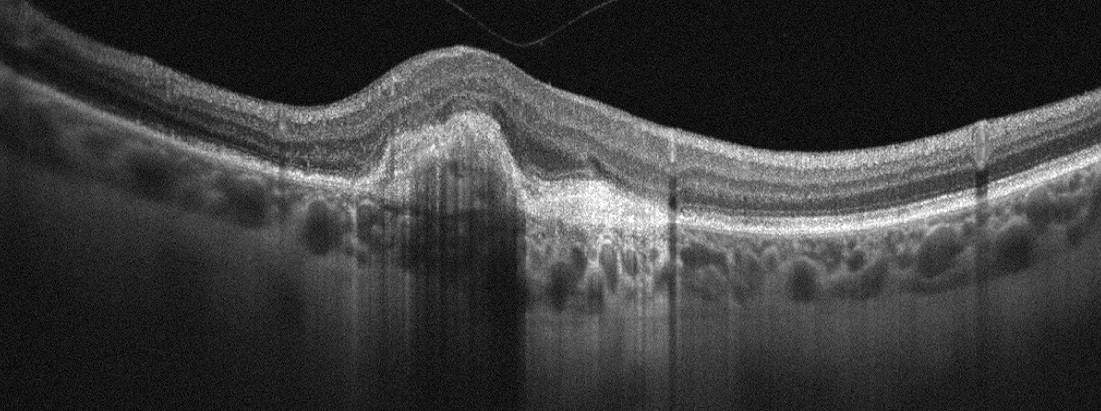
Optical coherence tomography scan.
Diagnosis: age-related macular degeneration (AMD).